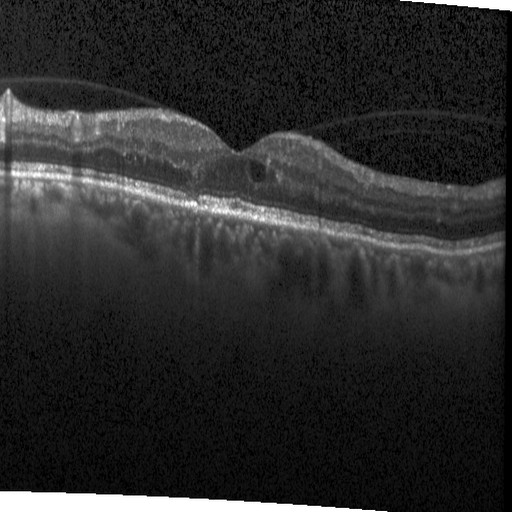 OCT B-scan.
This B-scan demonstrates diabetic macular edema (DME).